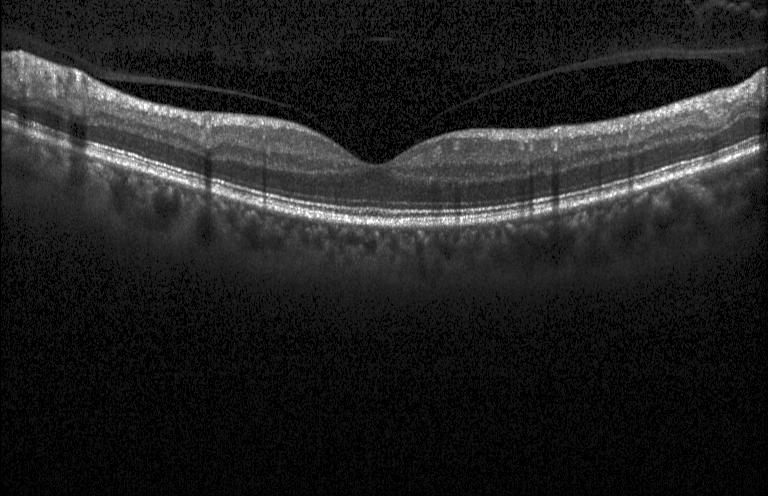
Optical coherence tomography scan. This B-scan demonstrates no choroidal neovascularization, no diabetic macular edema, and no drusen.